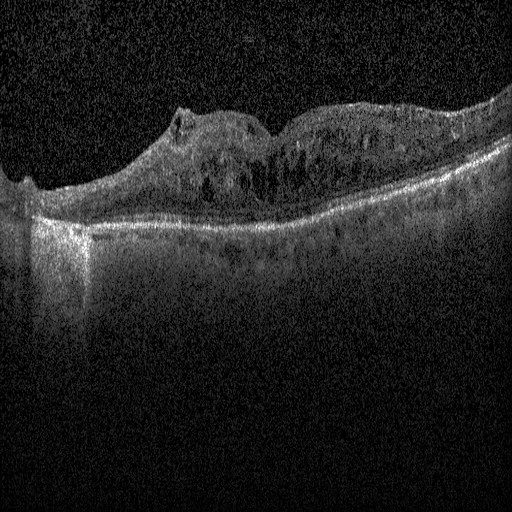

Fovea-centered · retinal OCT cross-section · SD-OCT · acquired on a Heidelberg Spectralis.
The scan shows diabetic macular edema (DME).